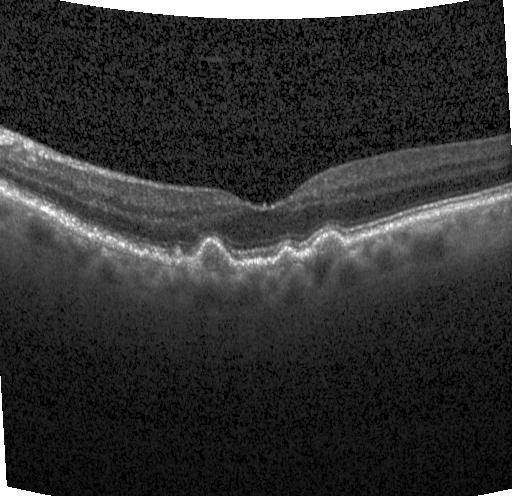
Retinal OCT B-scan.
Finding: drusen.